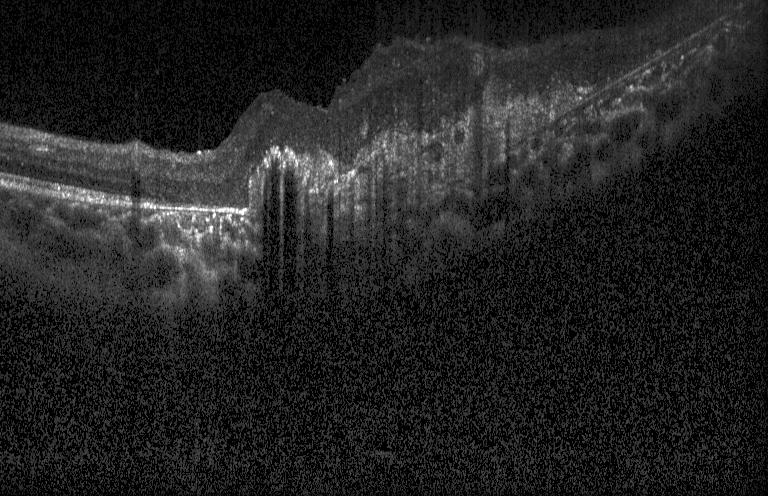 OCT B-scan — Macular OCT: choroidal neovascularization.